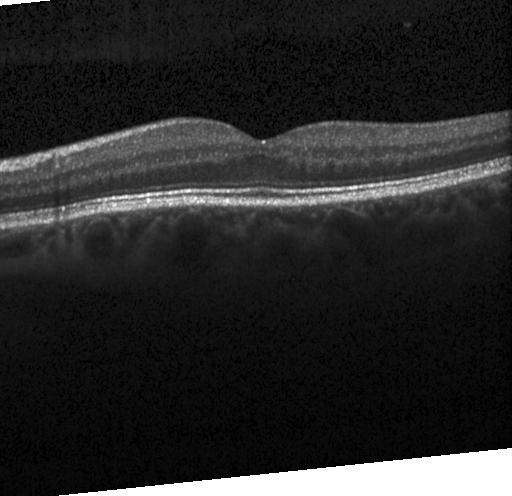 Retinal OCT cross-section
Assessment: no evidence of choroidal neovascularization, diabetic macular edema, or drusen.